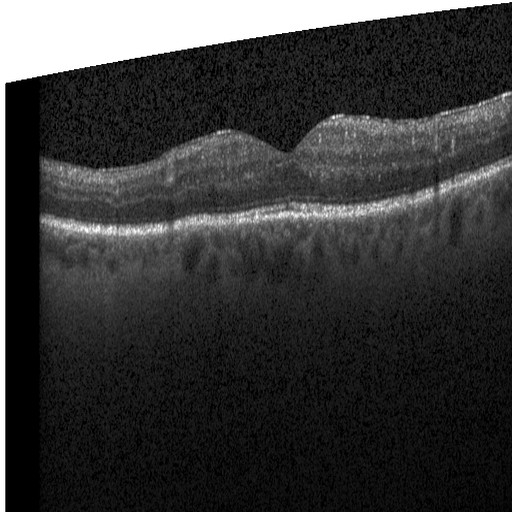 SD-OCT. Retinal OCT B-scan. Through the macula — This B-scan demonstrates DME.